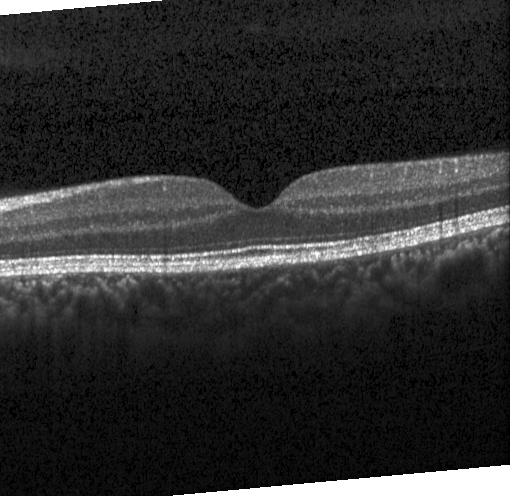
SD-OCT · Heidelberg Spectralis · OCT B-scan · through the macula. Diagnosis: neither choroidal neovascularization, diabetic macular edema, nor drusen.